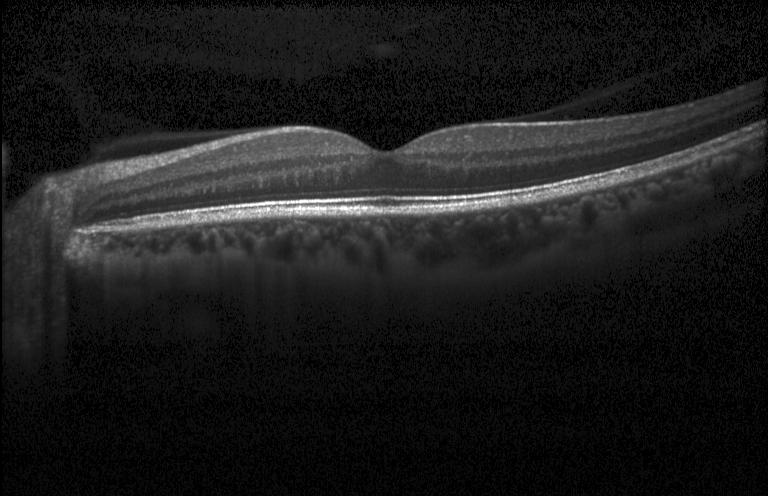
Optical coherence tomography scan.
This B-scan demonstrates no evidence of choroidal neovascularization, diabetic macular edema, or drusen.